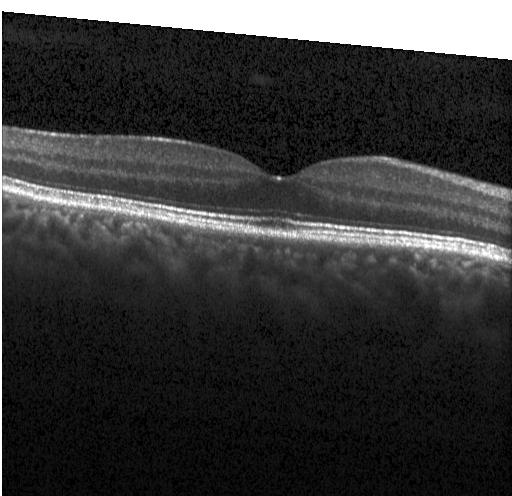

Heidelberg Spectralis, through the macula, OCT line scan, spectral-domain optical coherence tomography — Assessment: no CNV, DME, or drusen.